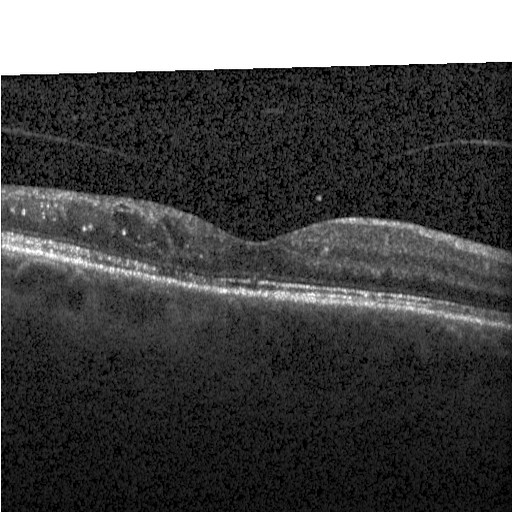
Spectral-domain optical coherence tomography. Optical coherence tomography scan — This B-scan demonstrates diabetic macular edema (DME).